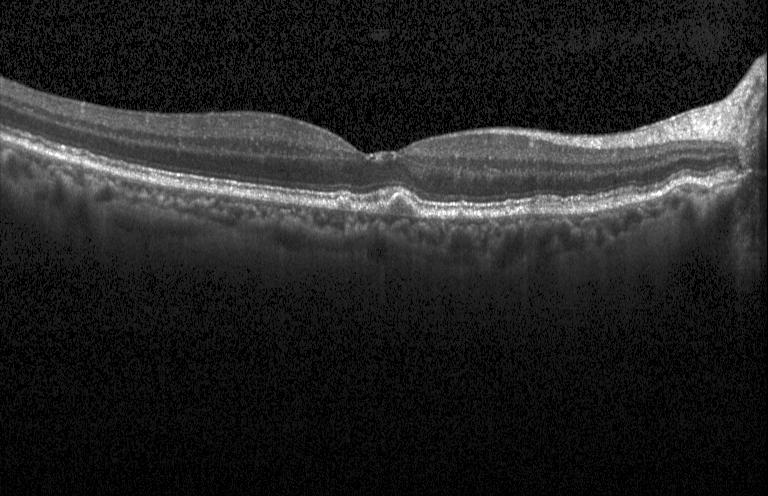

Retinal OCT cross-section showing drusen.